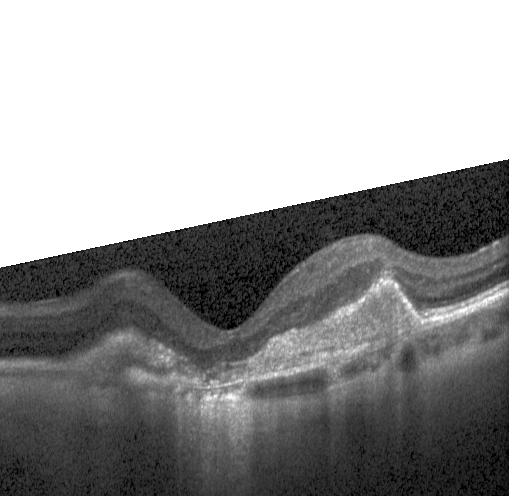

Optical coherence tomography B-scan. Acquired on a Heidelberg Spectralis. Spectral-domain optical coherence tomography. The scan shows CNV.